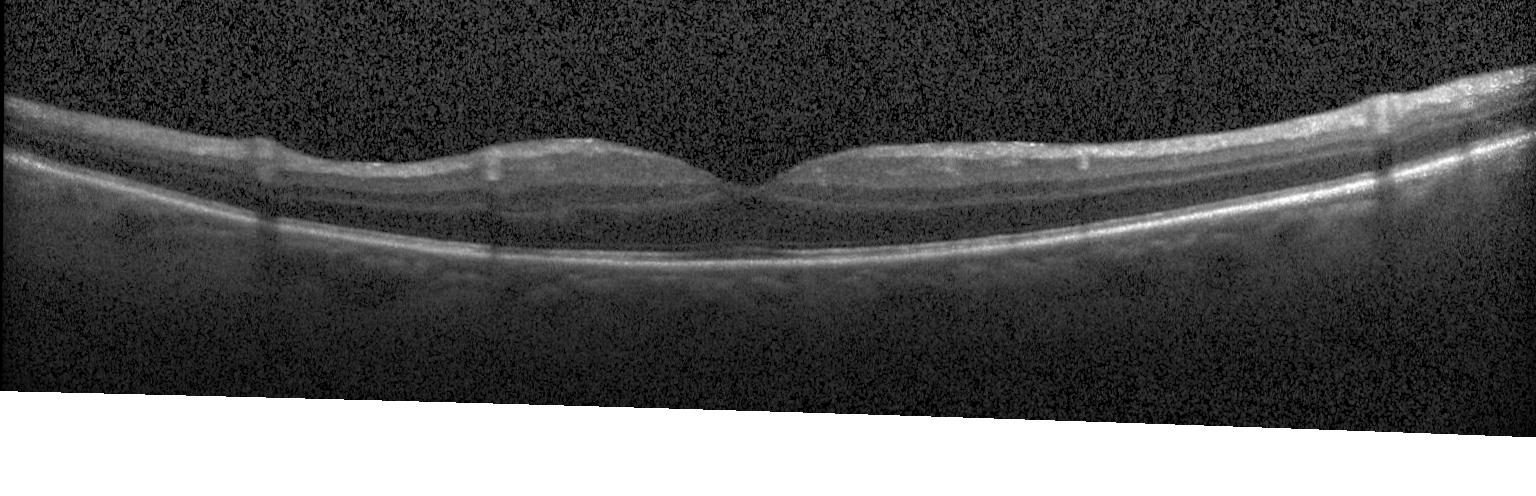 Heidelberg Spectralis OCT system, spectral-domain optical coherence tomography, through the macula, OCT B-scan — Diagnosis: no evidence of choroidal neovascularization, diabetic macular edema, or drusen.